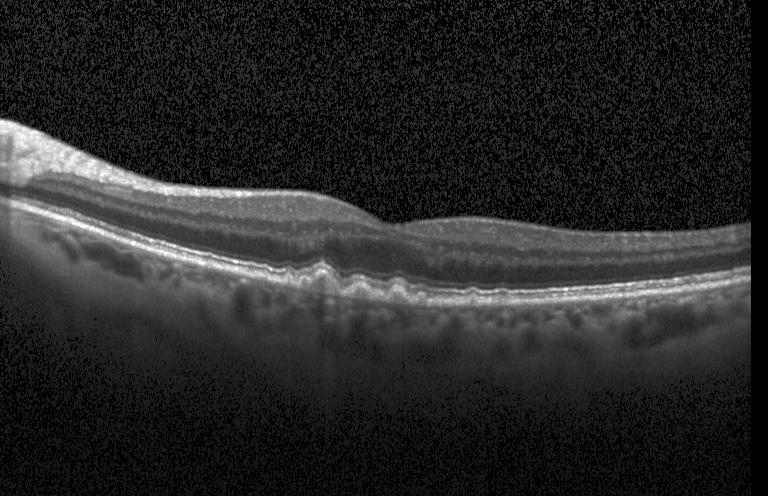 Through the macula · spectral-domain optical coherence tomography · retinal OCT cross-section — This B-scan demonstrates drusen.